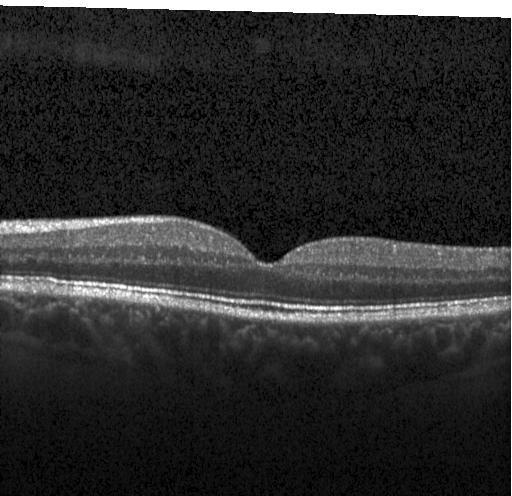

Macular OCT: no evidence of CNV, DME, or drusen.